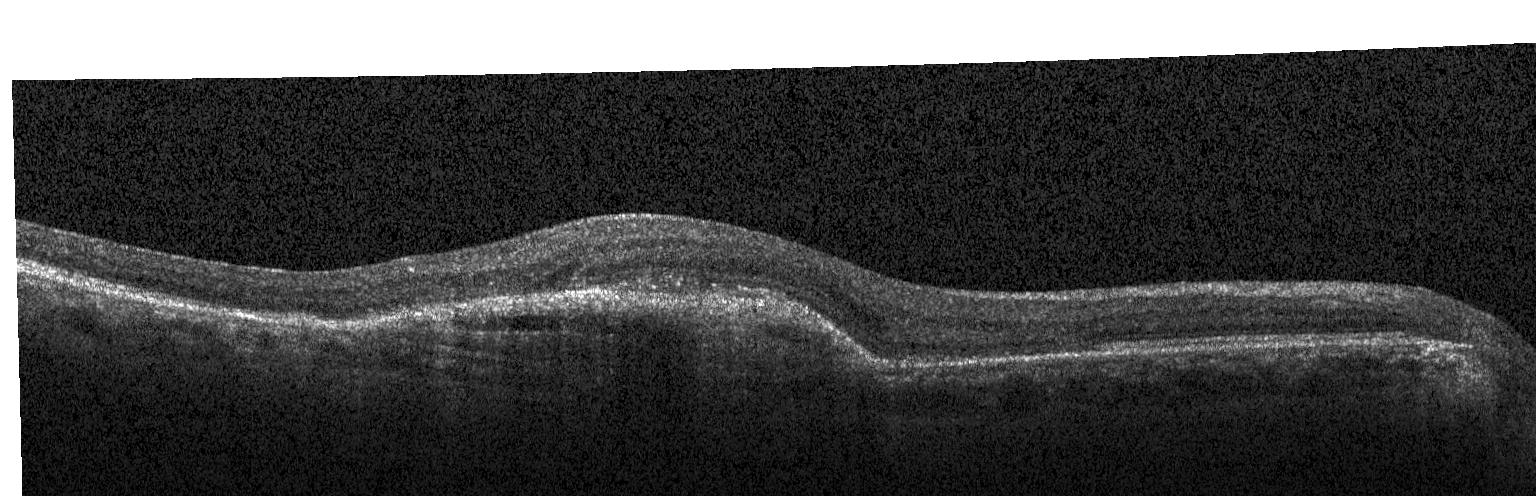
Impression: choroidal neovascularization.